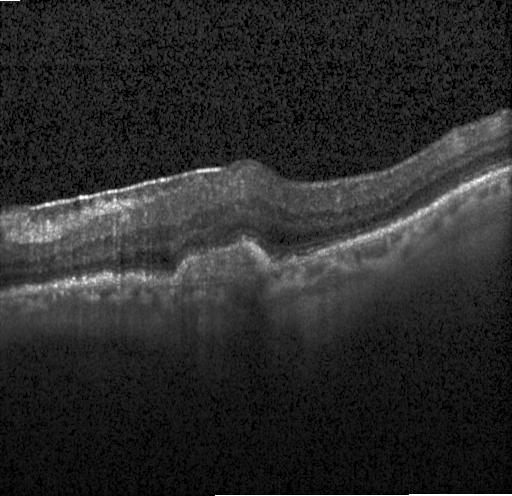 Finding: choroidal neovascularization.